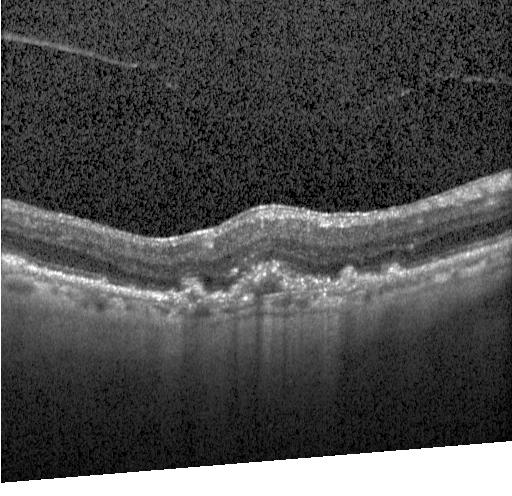 Retinal OCT cross-section
Diagnosis: a choroidal neovascular membrane.